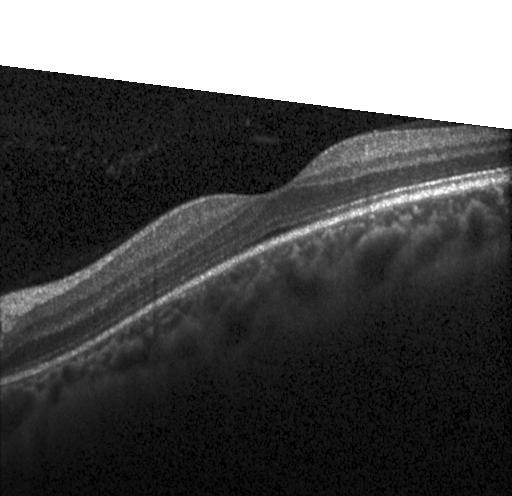 Fovea-centered, spectral-domain OCT, Heidelberg Spectralis, retinal OCT cross-section.
Dx: no evidence of choroidal neovascularization, diabetic macular edema, or drusen.